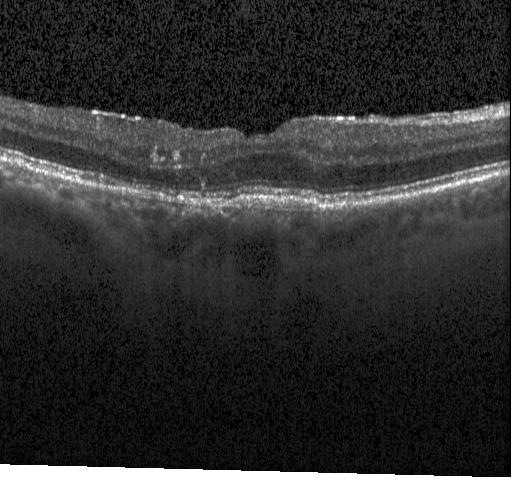 Impression: choroidal neovascularization.